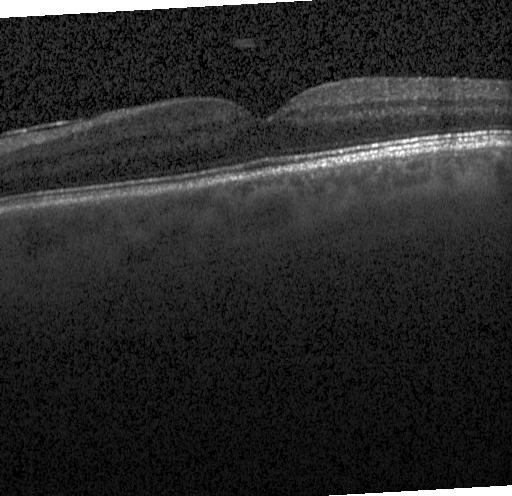
Impression: no evidence of CNV, DME, or drusen.